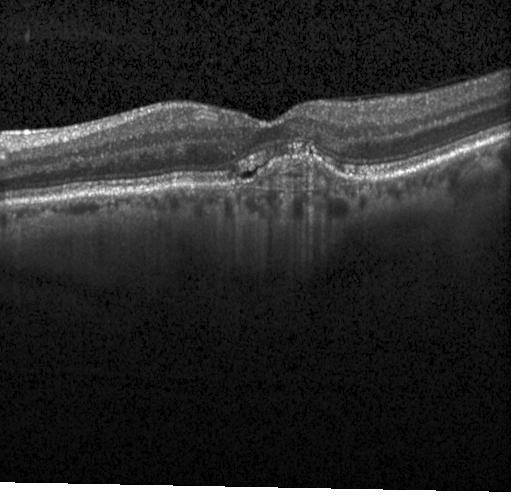
Retinal OCT B-scan, Heidelberg Spectralis OCT system, macular scan. The scan shows a choroidal neovascular membrane.